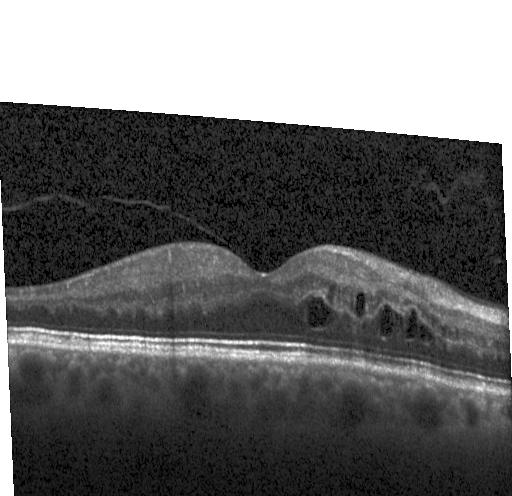
Heidelberg Spectralis OCT system. Centered on the fovea. Retinal OCT B-scan.
Finding: diabetic macular edema.